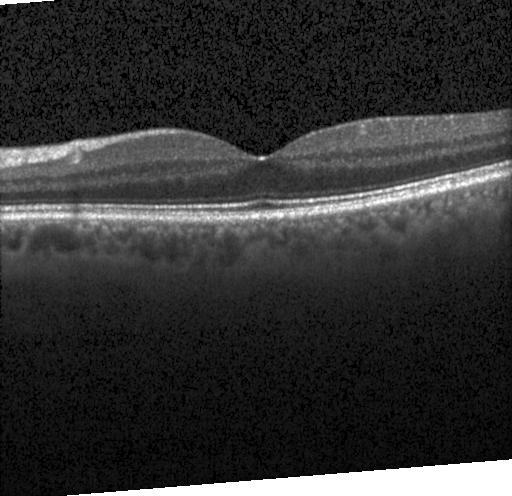 Diagnosis: no evidence of CNV, DME, or drusen.